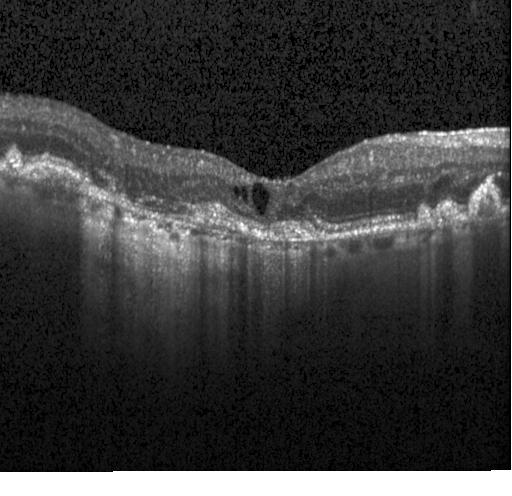
Optical coherence tomography scan. Instrument: Heidelberg Spectralis.
Impression: a choroidal neovascular membrane.